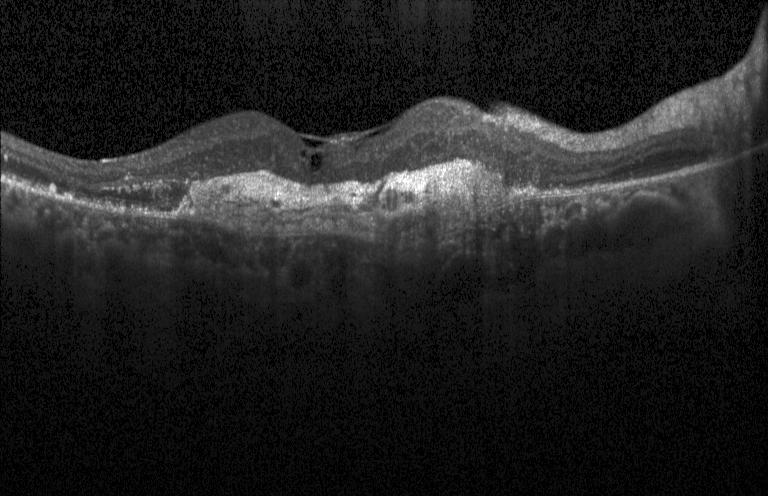

Impression: a choroidal neovascular membrane.